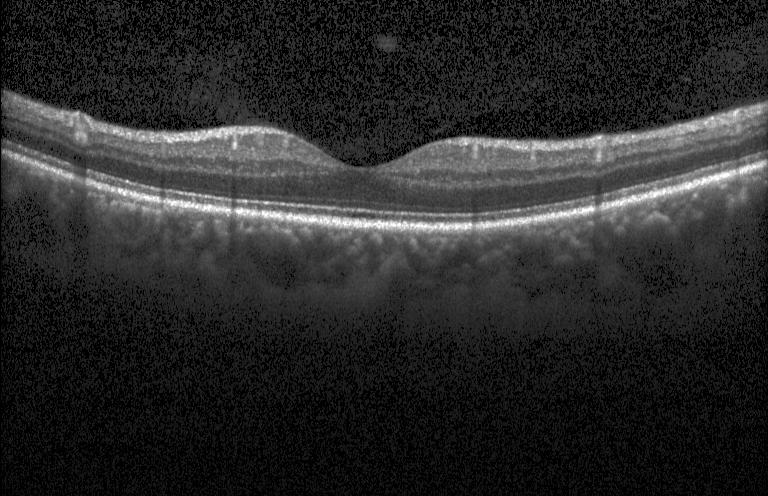

Finding: neither choroidal neovascularization, diabetic macular edema, nor drusen.